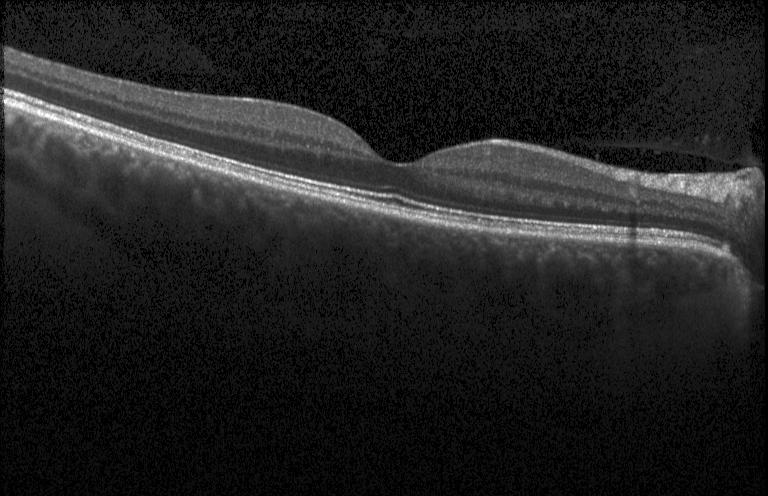

Macular OCT demonstrating no evidence of CNV, DME, or drusen.